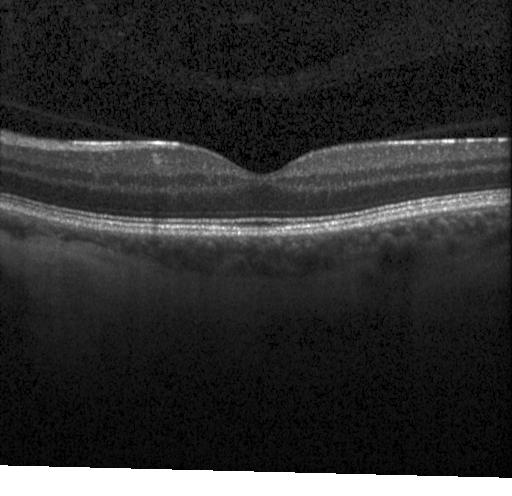
Macular OCT demonstrating no choroidal neovascularization, no diabetic macular edema, and no drusen.